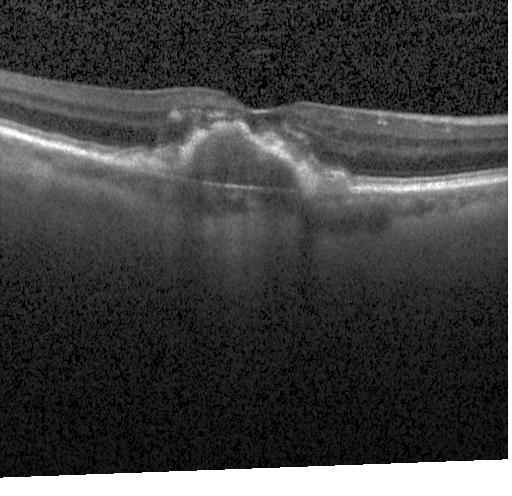

Instrument: Heidelberg Spectralis, OCT B-scan, through the macula, spectral-domain OCT. Diagnosis: CNV.